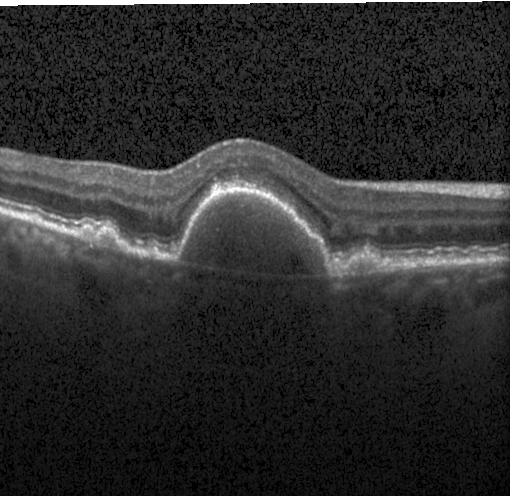
SD-OCT. Instrument: Heidelberg Spectralis. Retinal OCT B-scan. Centered on the fovea.
OCT finding: a choroidal neovascular membrane.